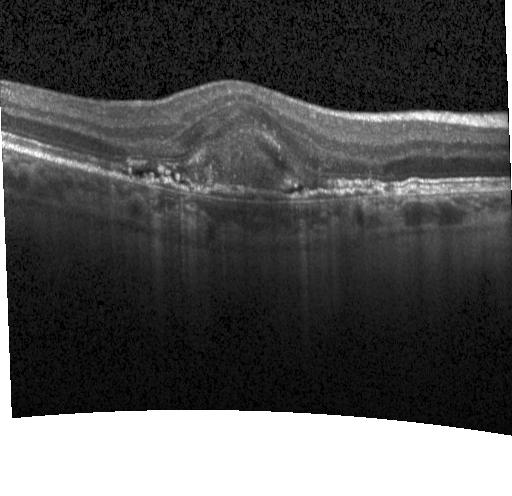 Spectral-domain OCT B-scan: choroidal neovascularization.